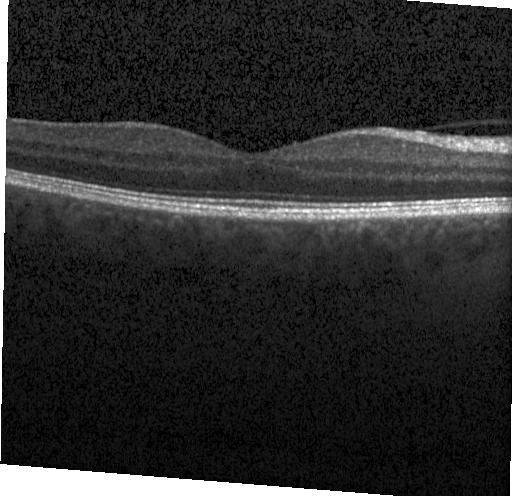
This B-scan demonstrates no evidence of choroidal neovascularization, diabetic macular edema, or drusen.